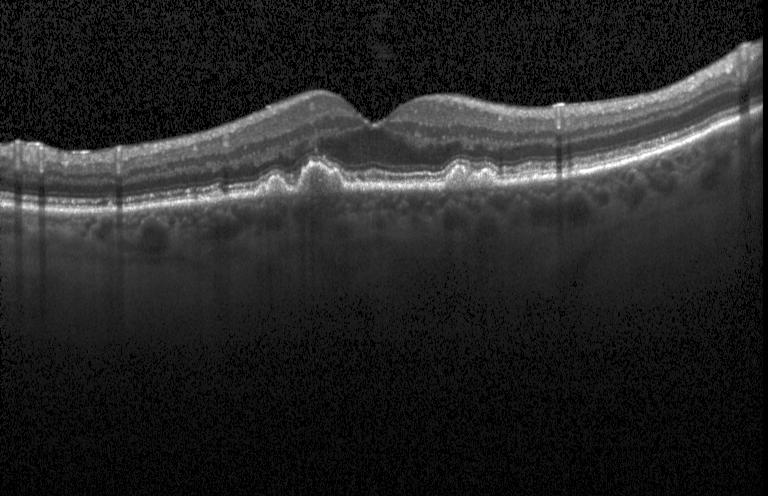 Spectral-domain OCT B-scan: sub-RPE drusenoid deposits.